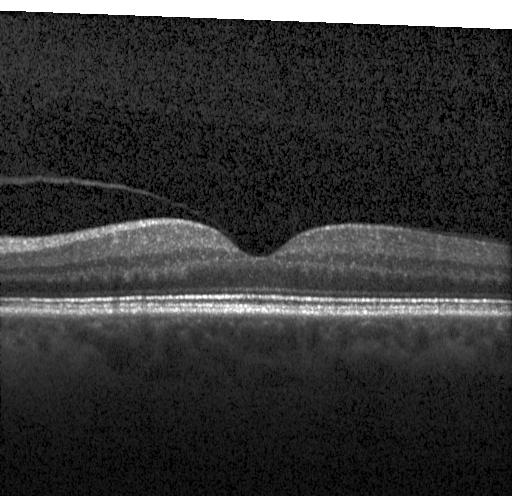 Optical coherence tomography B-scan
Assessment: no choroidal neovascularization, no diabetic macular edema, and no drusen.